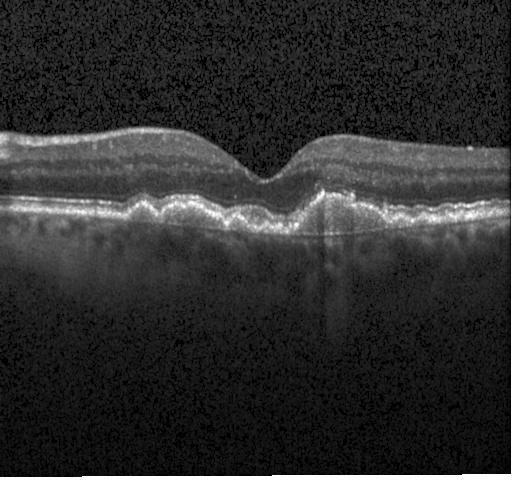 Heidelberg Spectralis; optical coherence tomography B-scan.
Macular OCT: multiple drusen.